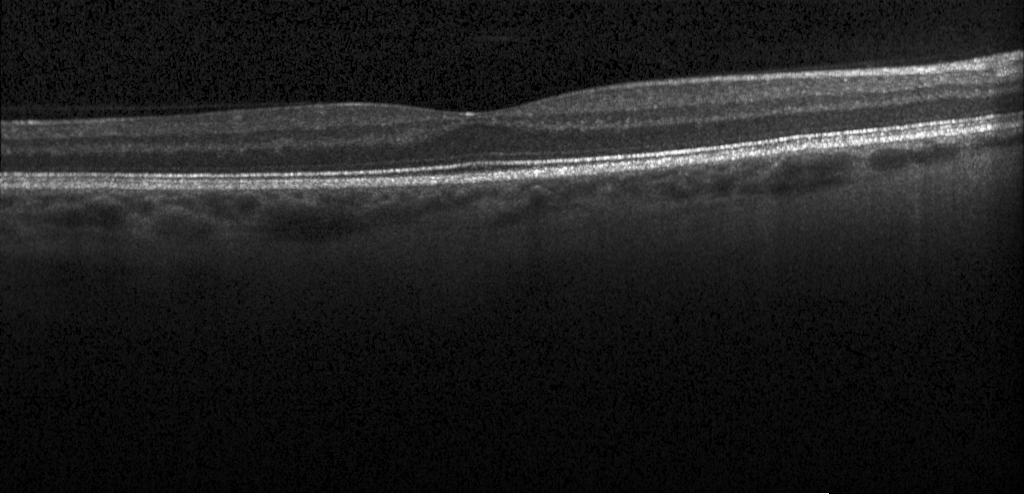

Impression: no CNV, DME, or drusen.